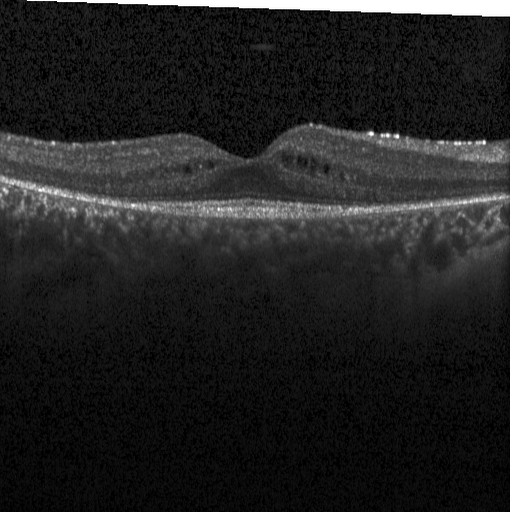 OCT scan showing diabetic macular edema (DME).